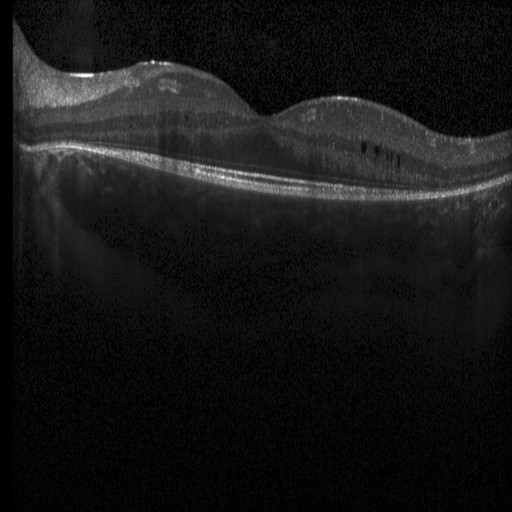

OCT line scan.
Finding: diabetic macular edema (DME).